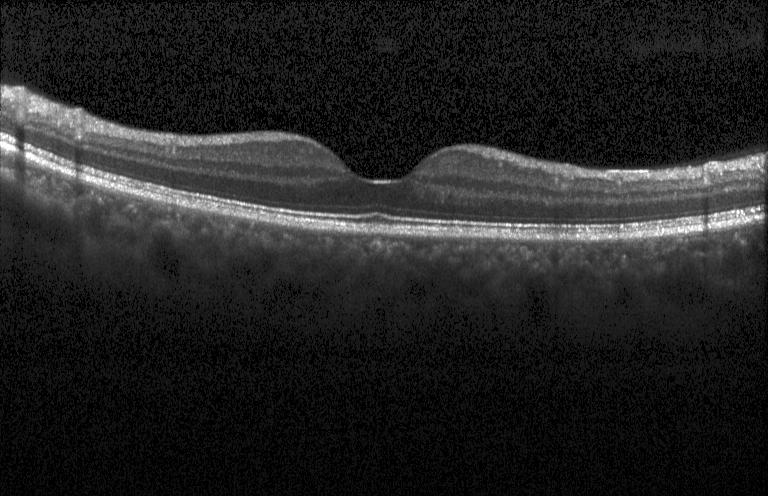 Diagnosis: no evidence of choroidal neovascularization, diabetic macular edema, or drusen.